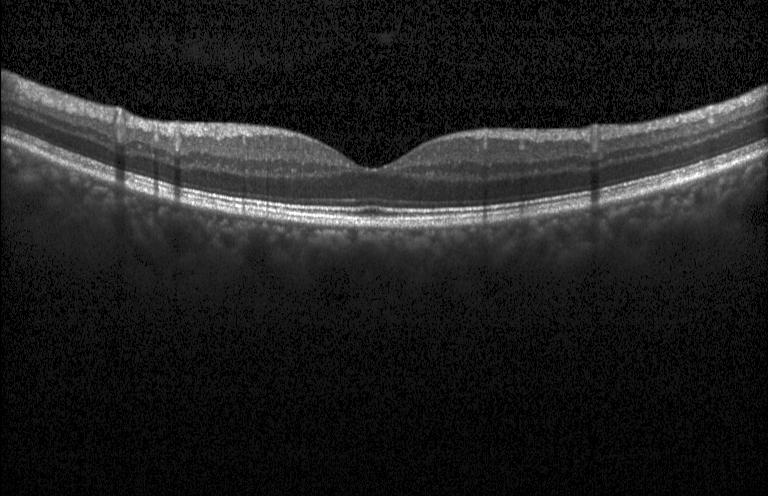 OCT B-scan. No evidence of choroidal neovascularization, diabetic macular edema, or drusen.